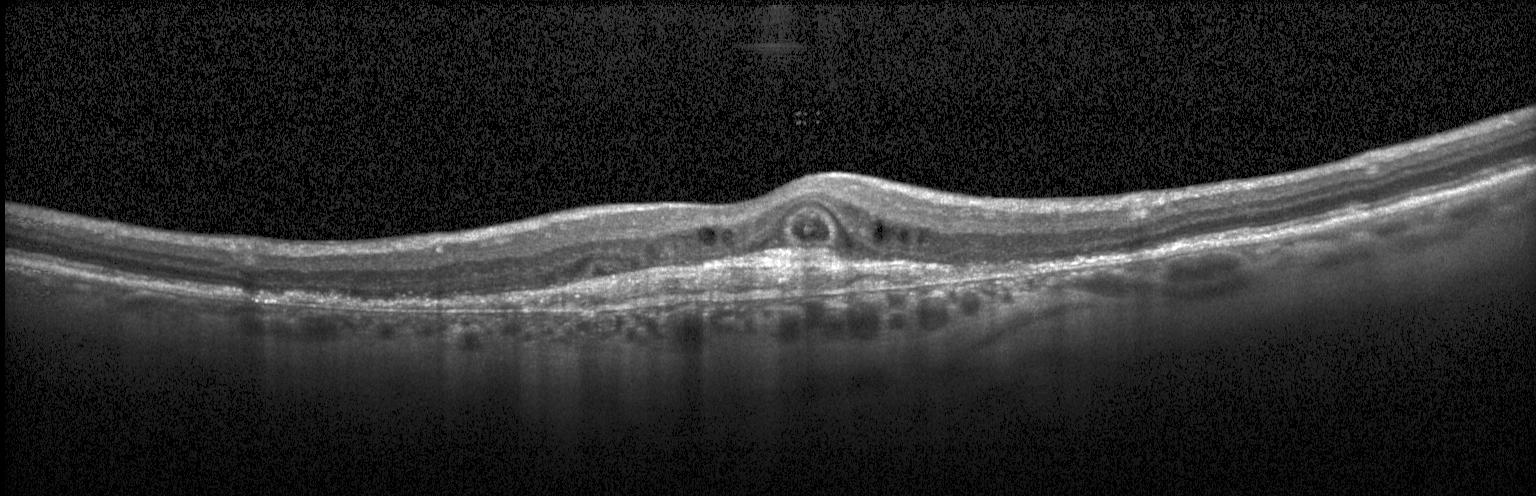 OCT scan showing choroidal neovascularization (CNV).